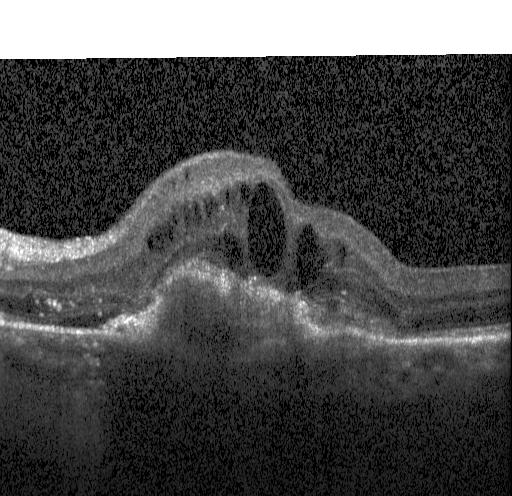 OCT B-scan.
Finding: choroidal neovascularization.